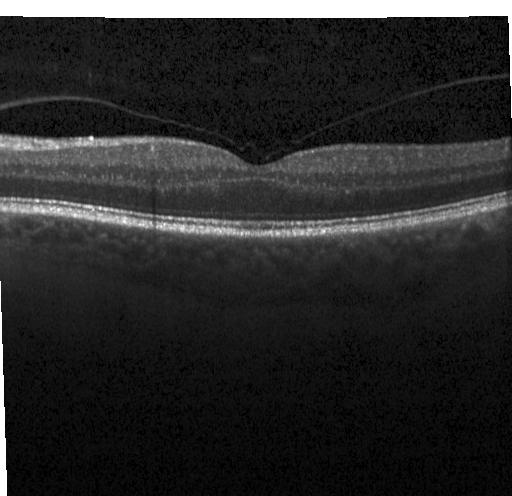 Centered on the fovea. Heidelberg Spectralis. Spectral-domain optical coherence tomography. Optical coherence tomography B-scan. OCT finding: no evidence of choroidal neovascularization, diabetic macular edema, or drusen.